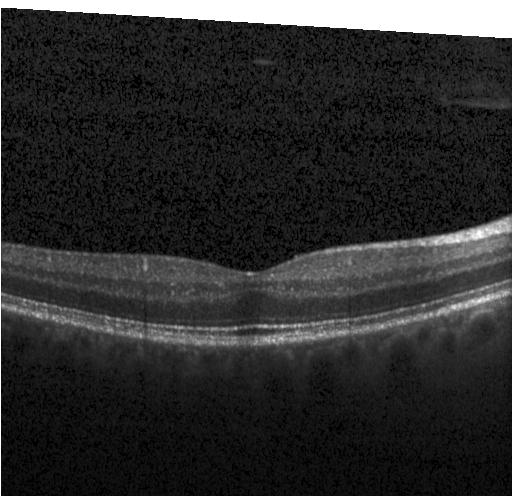
Macular OCT demonstrating no choroidal neovascularization, diabetic macular edema, or drusen.